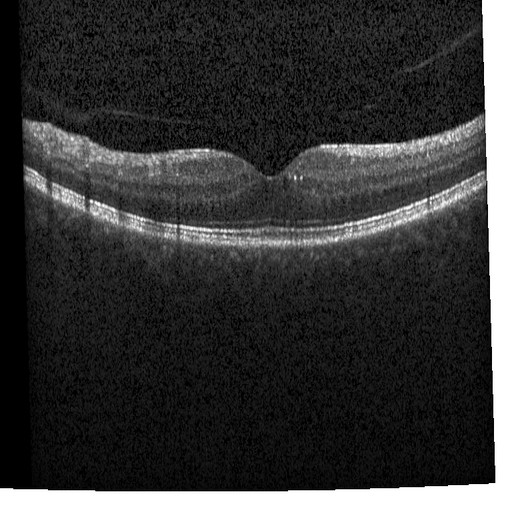 Retinal OCT cross-section; instrument: Heidelberg Spectralis.
Finding: diabetic macular edema (DME).